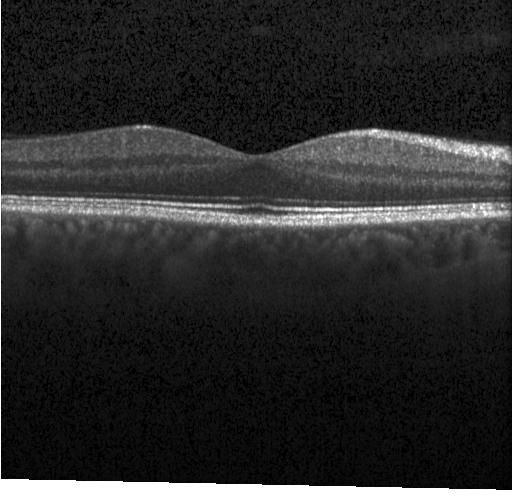
Instrument: Heidelberg Spectralis, fovea-centered, spectral-domain OCT, optical coherence tomography B-scan.
Neither choroidal neovascularization, diabetic macular edema, nor drusen.